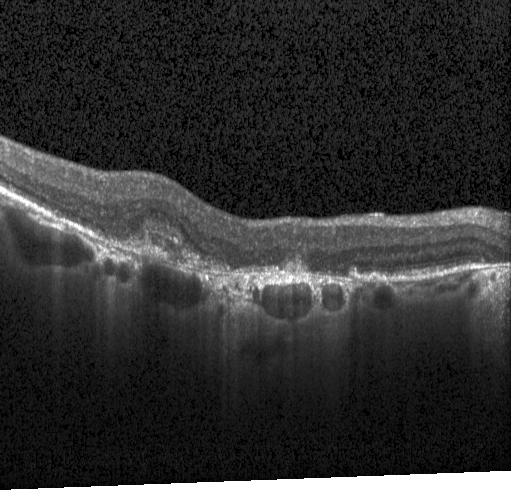

Macular scan, acquired on a Heidelberg Spectralis, SD-OCT, OCT line scan. Diagnosis: choroidal neovascularization.